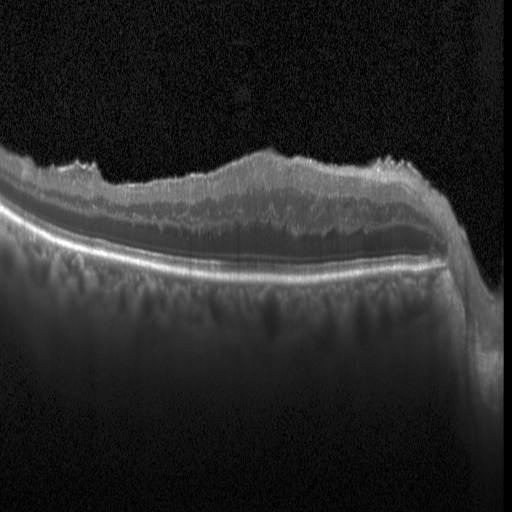
Acquired on a Heidelberg Spectralis; SD-OCT; optical coherence tomography scan.
Finding: diabetic macular edema (DME).